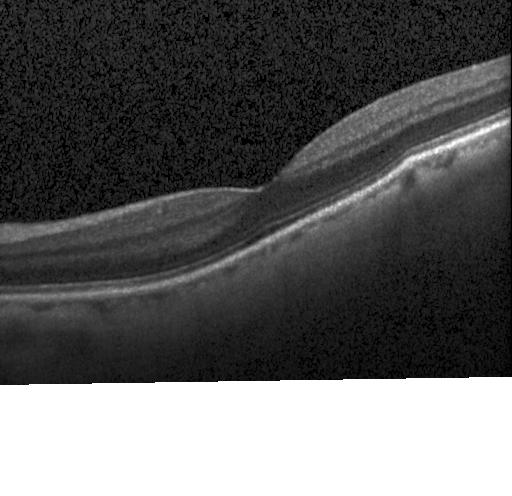

Optical coherence tomography B-scan
The scan shows neither CNV, DME, nor drusen.